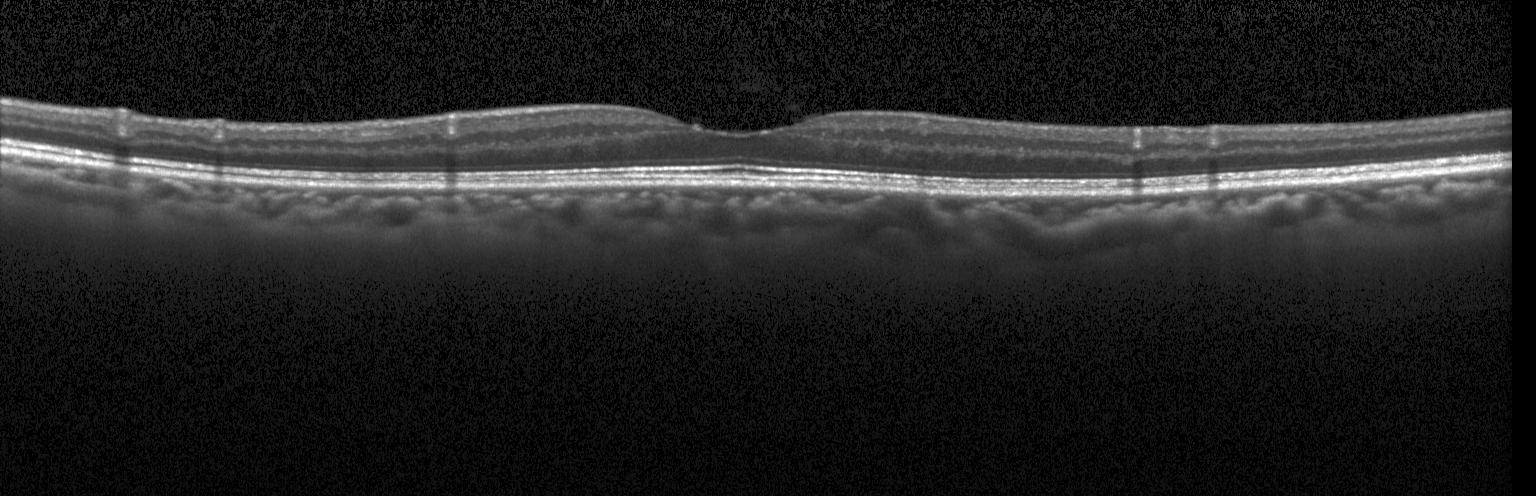

Optical coherence tomography B-scan
Finding: neither CNV, DME, nor drusen.